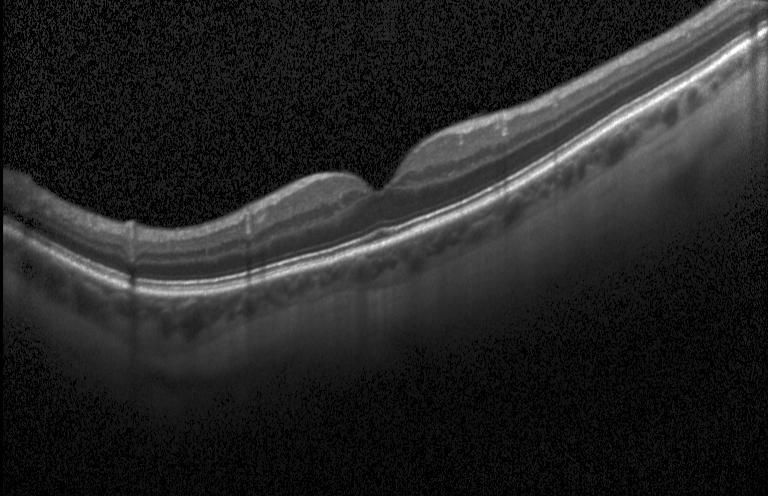

OCT B-scan · SD-OCT
Finding: neither choroidal neovascularization, diabetic macular edema, nor drusen.